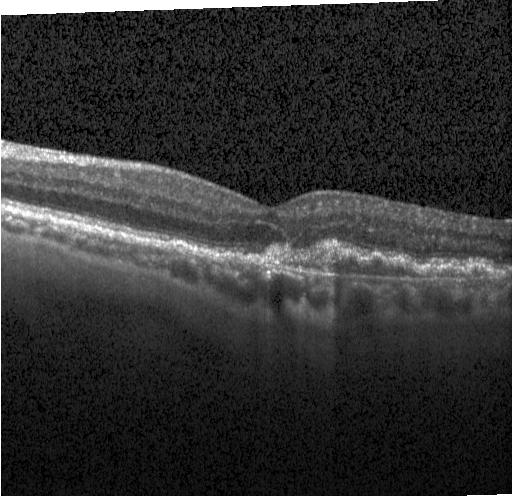
Finding: a choroidal neovascular membrane.